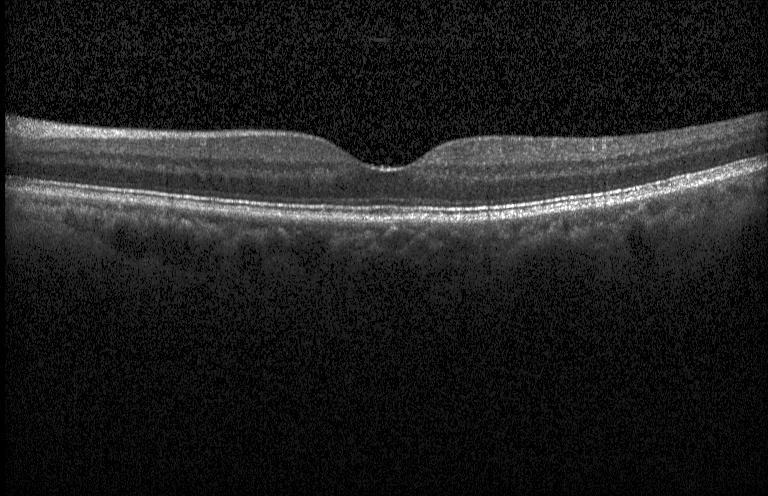 Optical coherence tomography scan. SD-OCT. Instrument: Heidelberg Spectralis. Through the macula.
Macular OCT: no evidence of choroidal neovascularization, diabetic macular edema, or drusen.